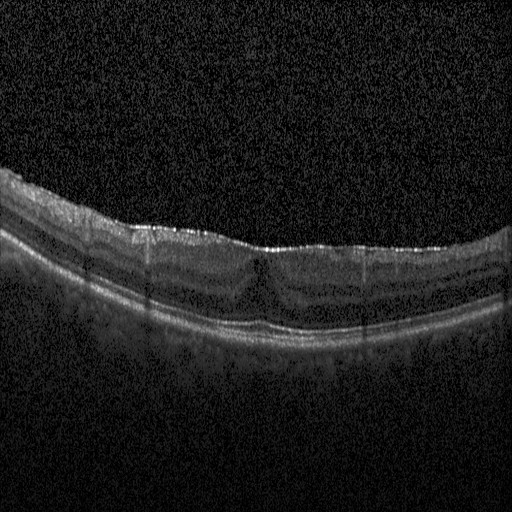
Diagnosis: diabetic macular edema.